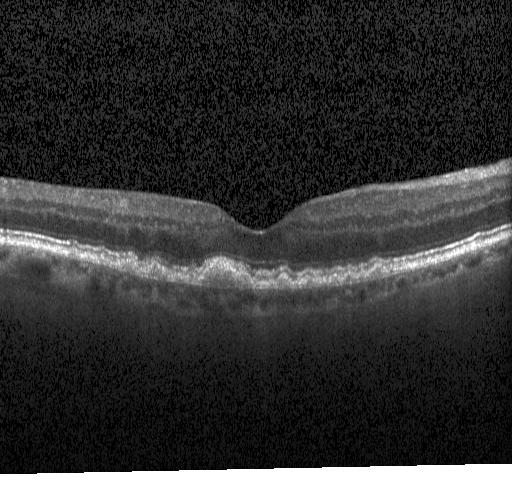 Horizontal scan through the fovea, acquired on a Heidelberg Spectralis, OCT line scan — Assessment: drusen.